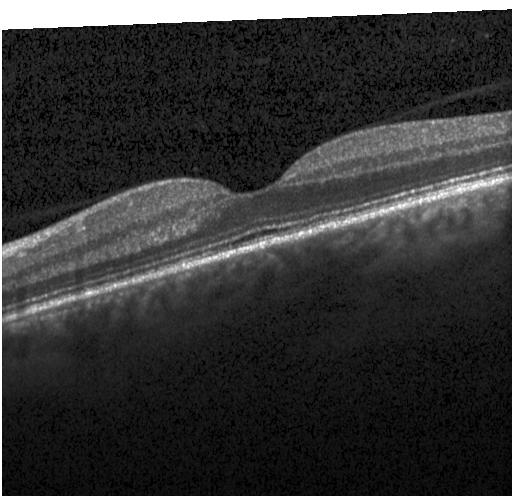
Retinal OCT B-scan — Impression: no choroidal neovascularization, diabetic macular edema, or drusen.